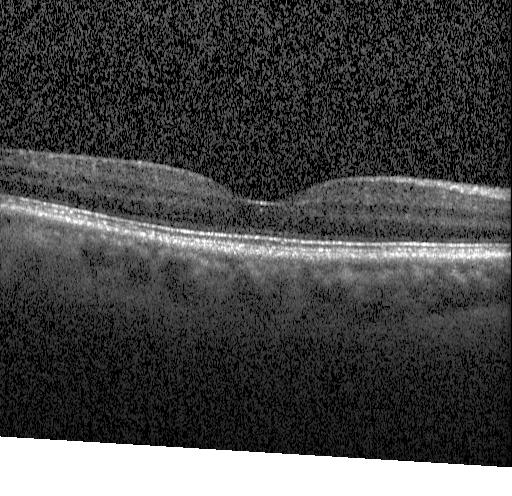

OCT B-scan. Finding: no choroidal neovascularization, diabetic macular edema, or drusen.